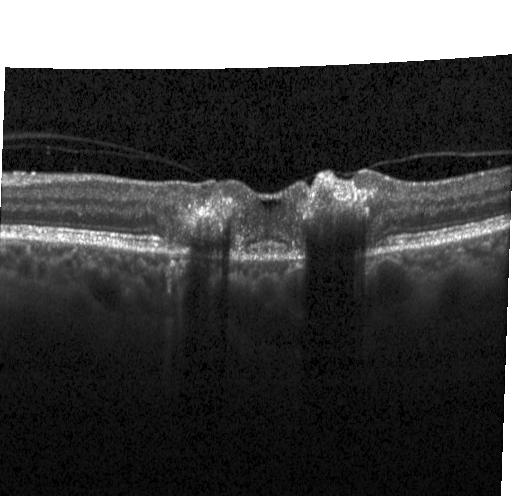 Finding: a choroidal neovascular membrane.